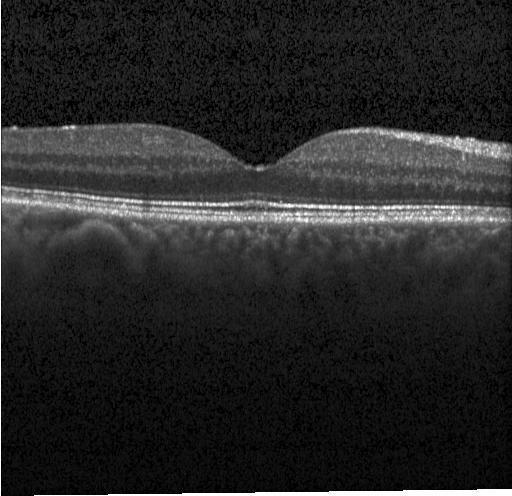 Spectral-domain optical coherence tomography; optical coherence tomography B-scan; centered on the fovea; instrument: Heidelberg Spectralis. Diagnosis: no CNV, DME, or drusen.